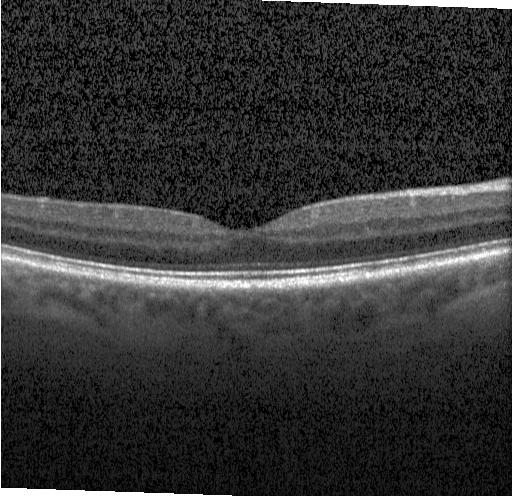 Macular OCT: no choroidal neovascularization, diabetic macular edema, or drusen.